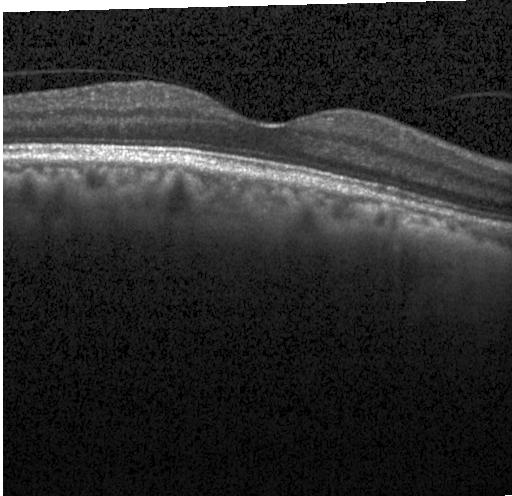
Heidelberg Spectralis OCT system, OCT line scan, spectral-domain optical coherence tomography. Impression: no choroidal neovascularization, diabetic macular edema, or drusen.